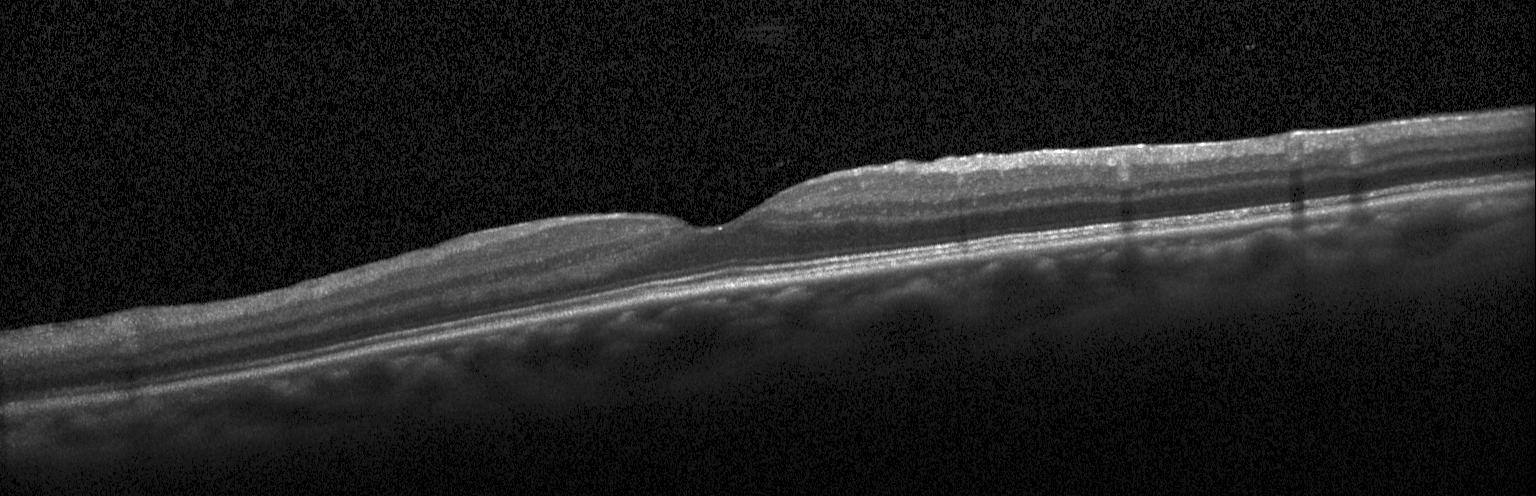 OCT line scan, horizontal scan through the fovea, Heidelberg Spectralis OCT system, SD-OCT.
OCT finding: no choroidal neovascularization, no diabetic macular edema, and no drusen.